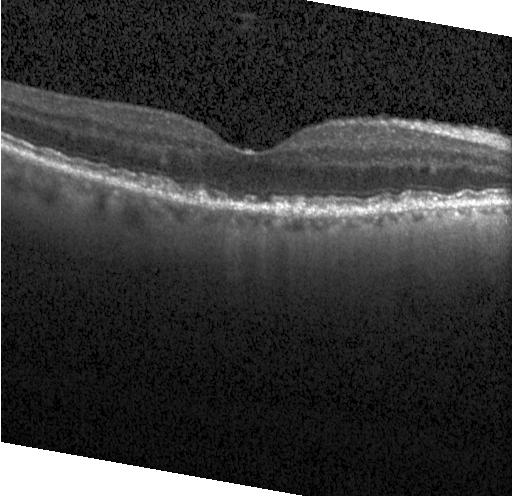
OCT B-scan showing multiple drusen.